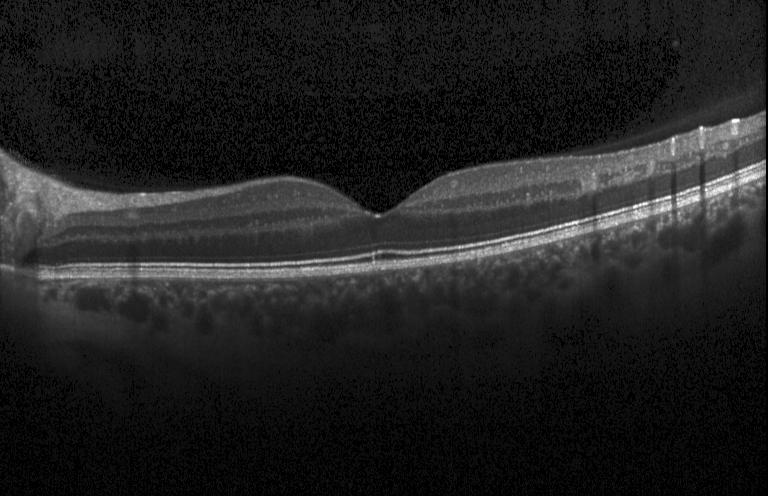
Dx: neither choroidal neovascularization, diabetic macular edema, nor drusen.